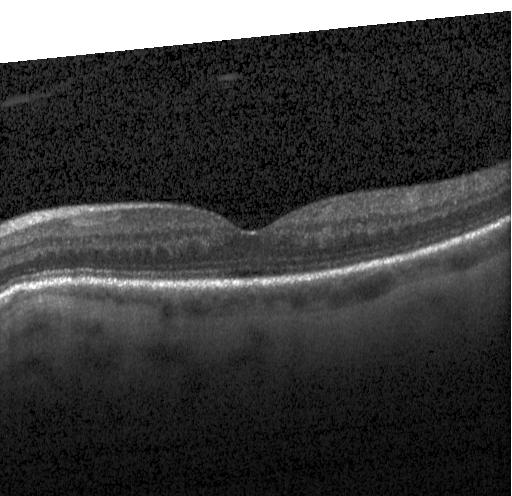 No choroidal neovascularization, no diabetic macular edema, and no drusen.